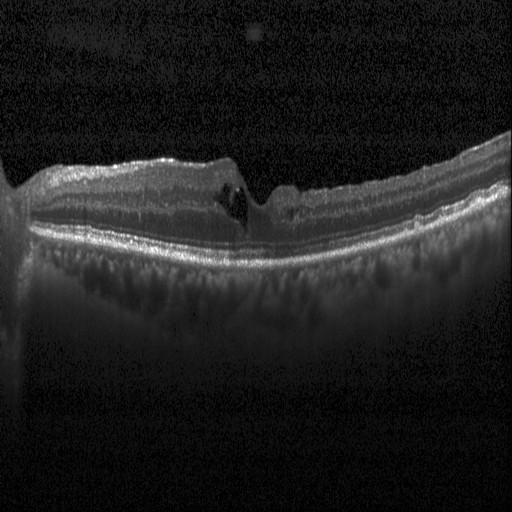
Retinal OCT B-scan. Heidelberg Spectralis OCT system
OCT finding: diabetic macular edema (DME).